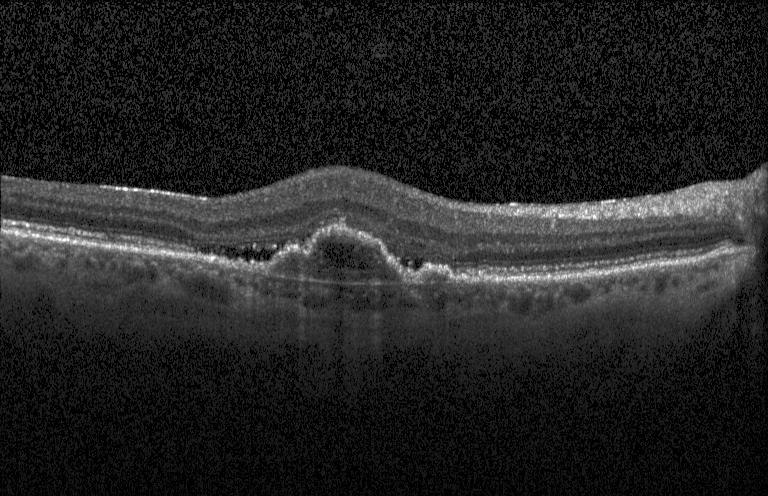 Optical coherence tomography B-scan; instrument: Heidelberg Spectralis; spectral-domain optical coherence tomography.
Macular OCT: choroidal neovascularization.